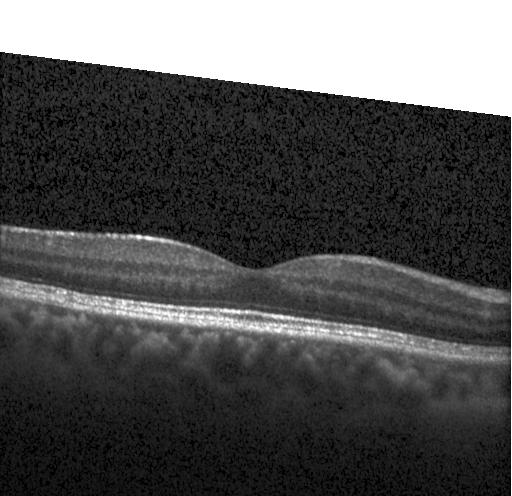
OCT B-scan. Macular scan.
This B-scan demonstrates neither choroidal neovascularization, diabetic macular edema, nor drusen.